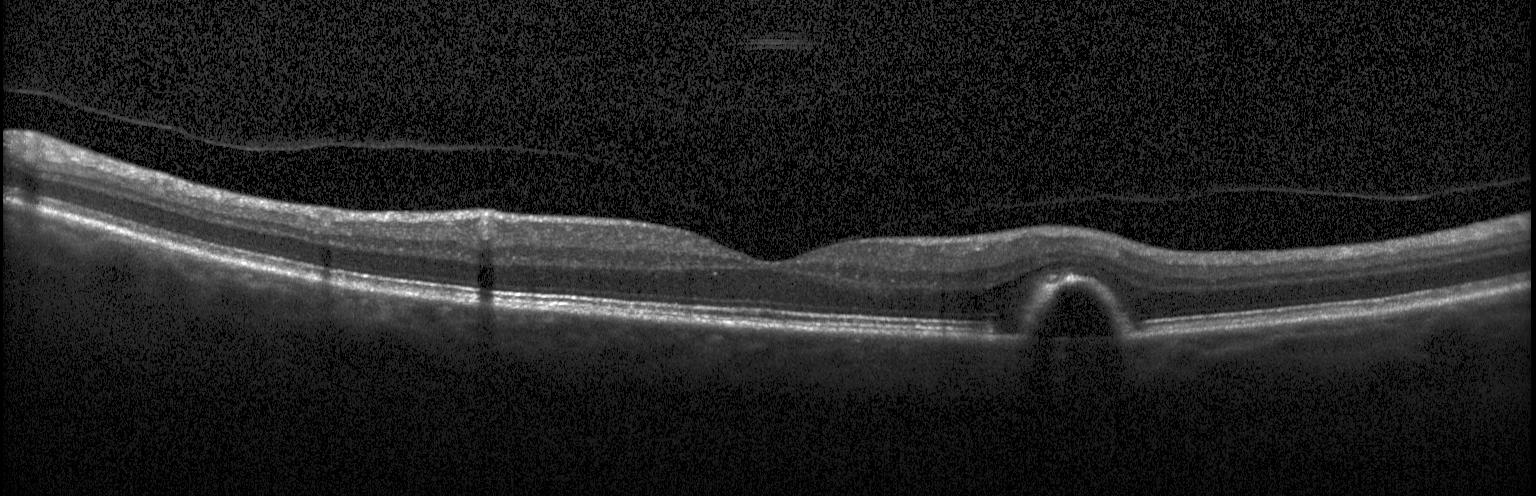
A choroidal neovascular membrane.